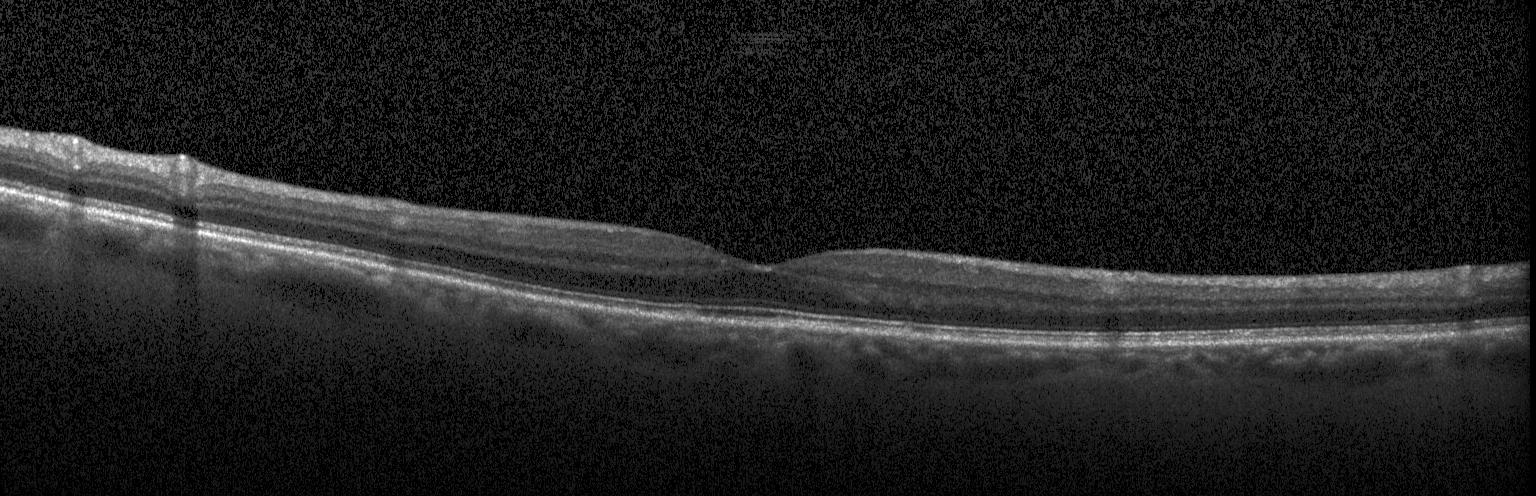
Optical coherence tomography scan · horizontal scan through the fovea · Heidelberg Spectralis · spectral-domain optical coherence tomography.
Dx: no choroidal neovascularization, no diabetic macular edema, and no drusen.